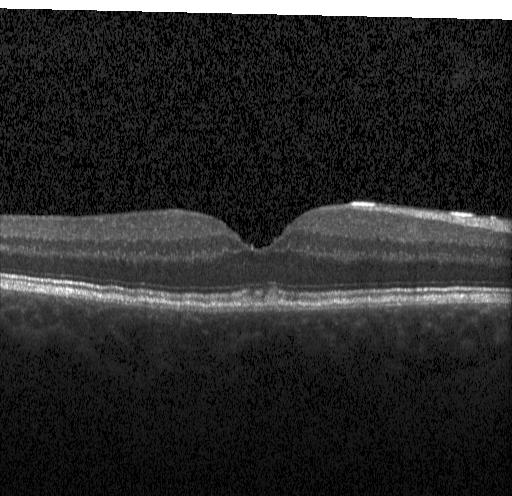

Macular scan; retinal OCT cross-section; spectral-domain OCT; acquired on a Heidelberg Spectralis
Drusen.